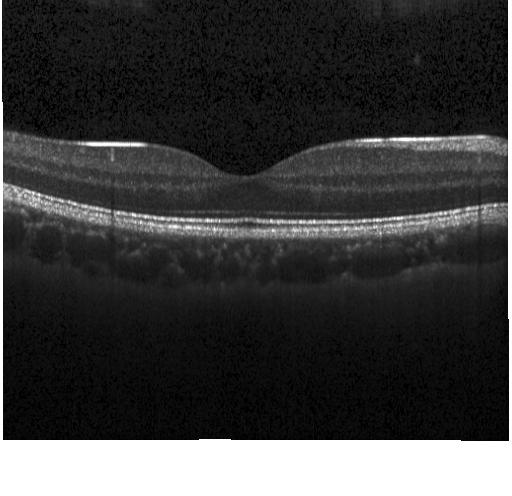

Macular OCT: no choroidal neovascularization, diabetic macular edema, or drusen.